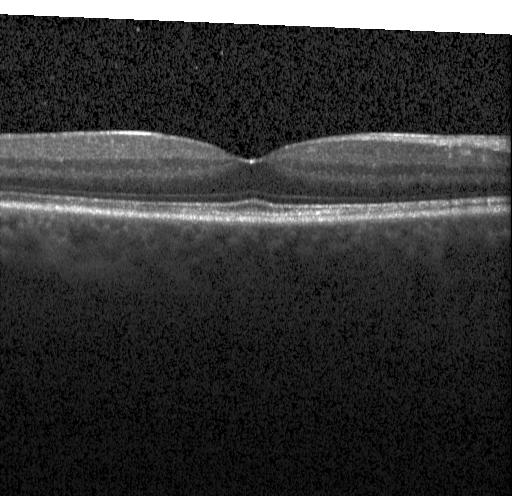 Finding: no evidence of choroidal neovascularization, diabetic macular edema, or drusen.